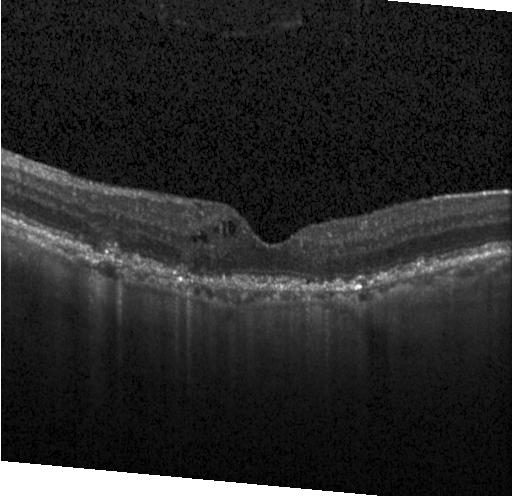 Through the macula, instrument: Heidelberg Spectralis, optical coherence tomography scan, SD-OCT. Impression: a choroidal neovascular membrane.